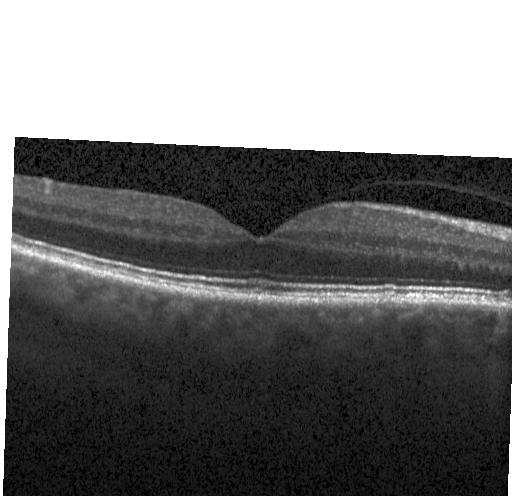
OCT B-scan. Impression: neither choroidal neovascularization, diabetic macular edema, nor drusen.